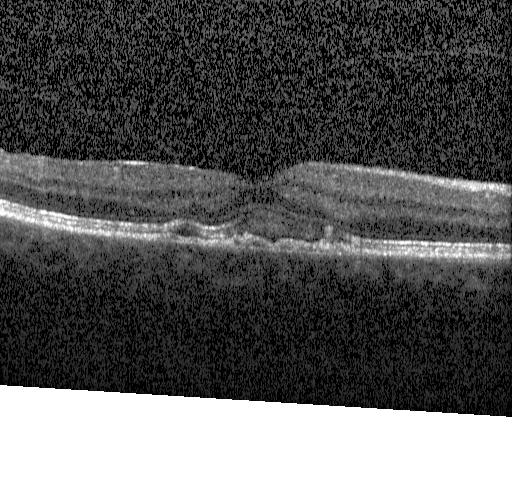
Spectral-domain OCT B-scan: a choroidal neovascular membrane.